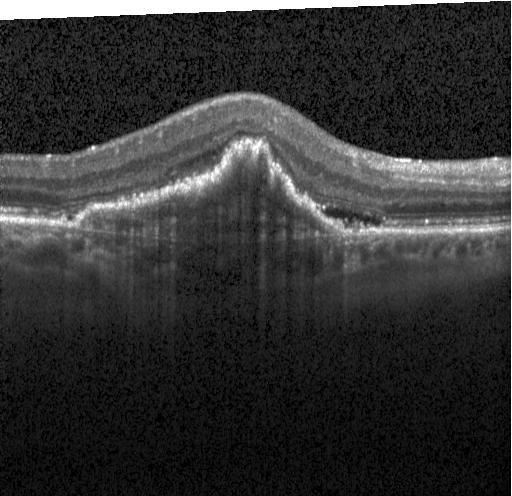
Spectral-domain optical coherence tomography. Acquired on a Heidelberg Spectralis. Optical coherence tomography scan. Centered on the fovea.
Impression: CNV.